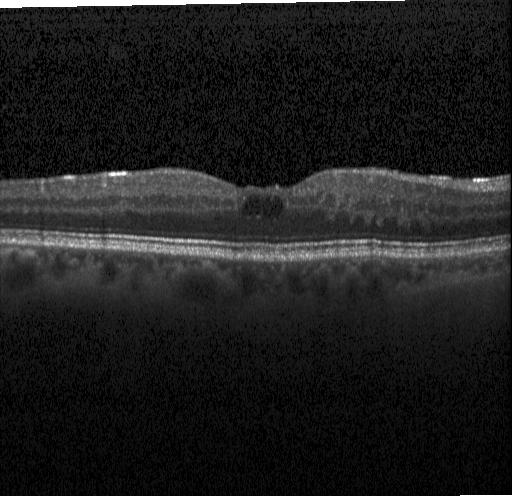

Diagnosis: DME.